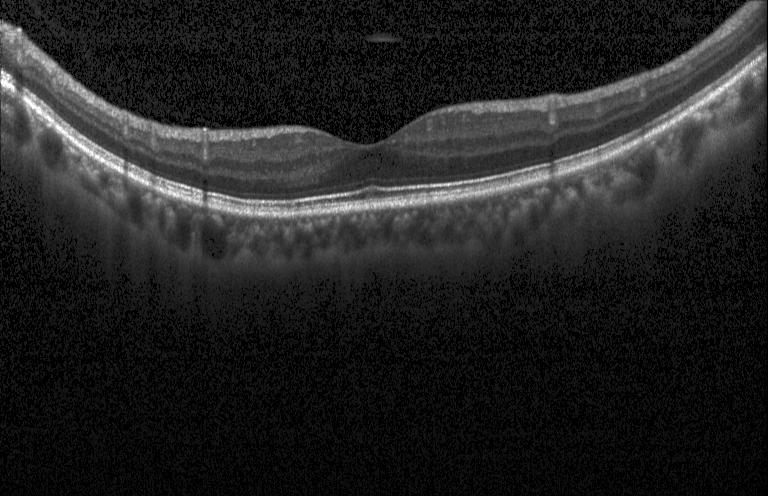
Optical coherence tomography B-scan.
Diagnosis: neither choroidal neovascularization, diabetic macular edema, nor drusen.